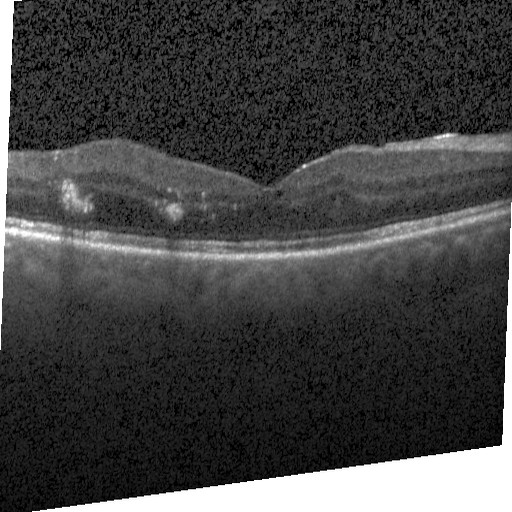 This B-scan demonstrates diabetic macular edema (DME).